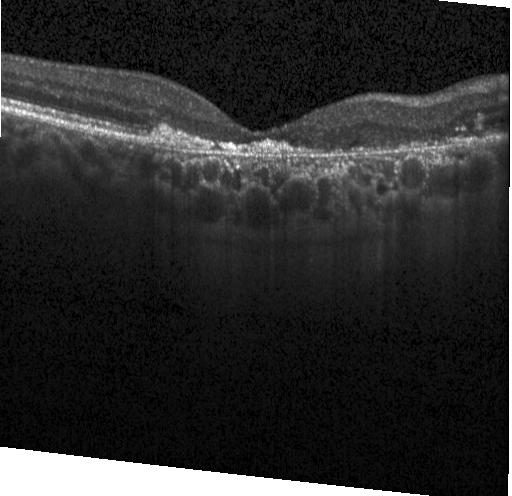

Macular OCT: a choroidal neovascular membrane.